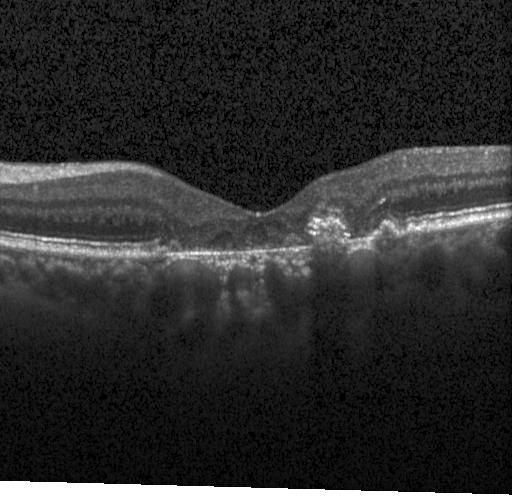 SD-OCT · horizontal scan through the fovea · optical coherence tomography scan — Diagnosis: a choroidal neovascular membrane.